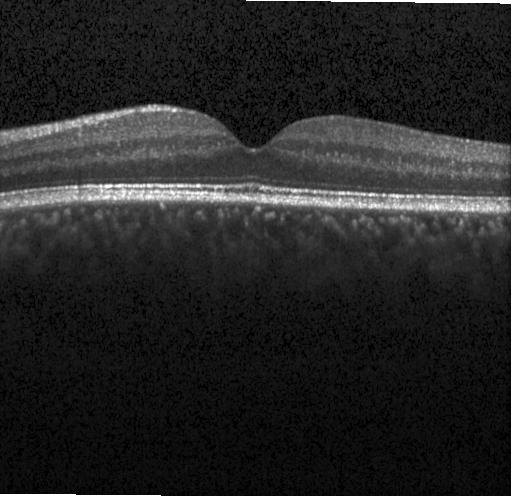
Optical coherence tomography scan, centered on the fovea — Assessment: no evidence of choroidal neovascularization, diabetic macular edema, or drusen.